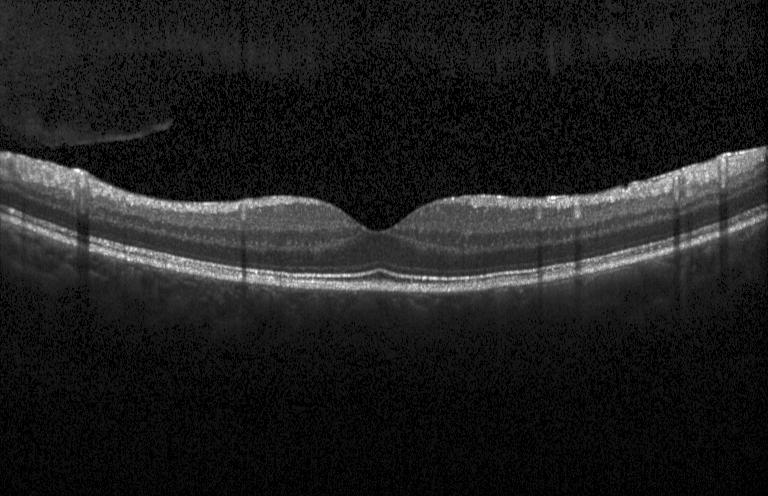

OCT B-scan
The scan shows no choroidal neovascularization, diabetic macular edema, or drusen.